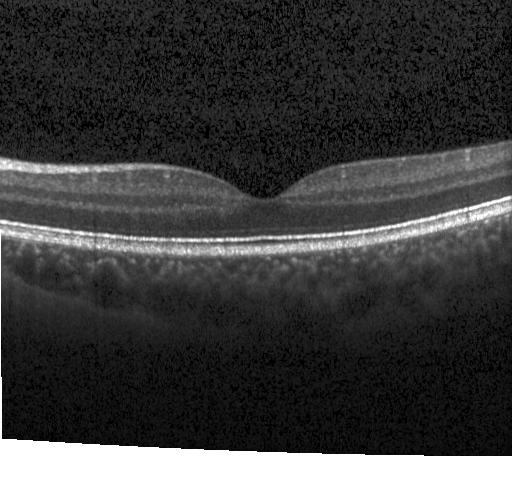

Optical coherence tomography scan, acquired on a Heidelberg Spectralis, SD-OCT, horizontal scan through the fovea — Macular OCT: neither choroidal neovascularization, diabetic macular edema, nor drusen.